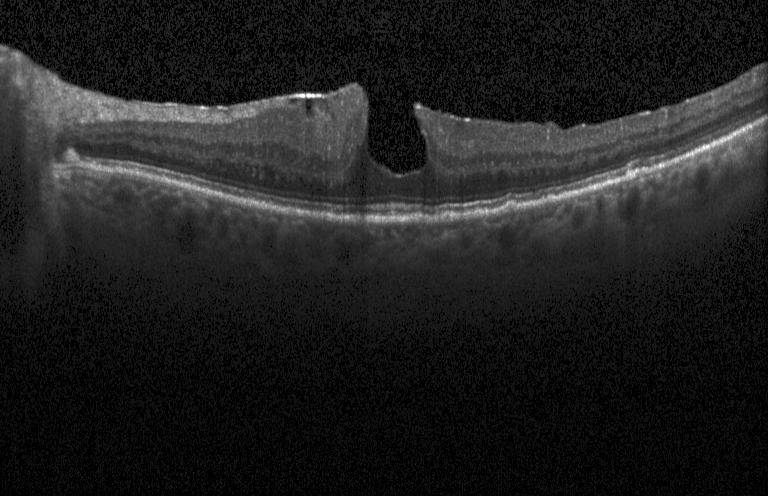 Instrument: Heidelberg Spectralis. OCT B-scan. SD-OCT. Macular scan. Diabetic macular edema (DME).